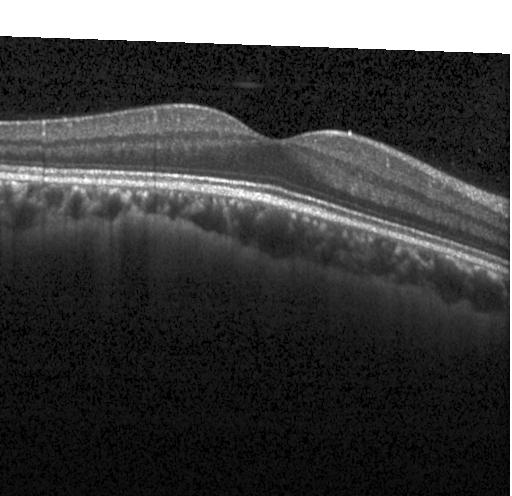

No CNV, DME, or drusen.